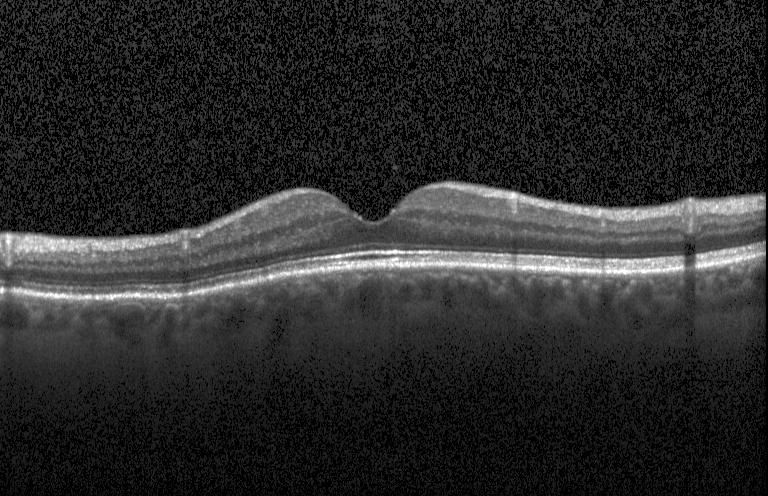
Fovea-centered · retinal OCT B-scan · SD-OCT · acquired on a Heidelberg Spectralis
Finding: no choroidal neovascularization, no diabetic macular edema, and no drusen.